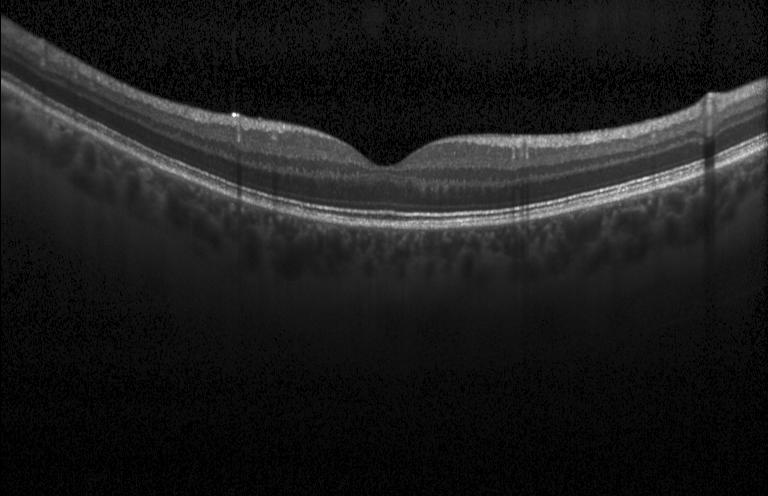
Instrument: Heidelberg Spectralis; SD-OCT; optical coherence tomography scan.
Impression: no evidence of choroidal neovascularization, diabetic macular edema, or drusen.